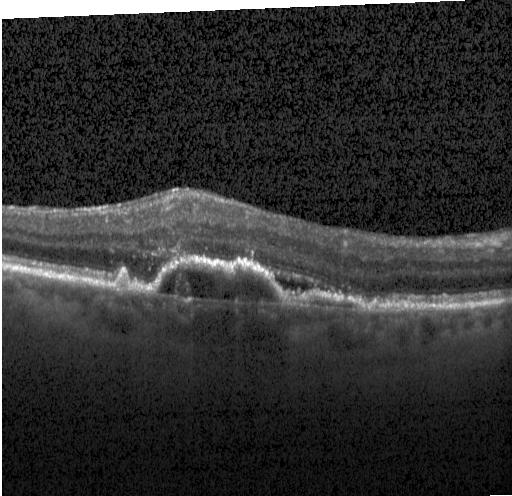
Optical coherence tomography scan
OCT finding: a choroidal neovascular membrane.